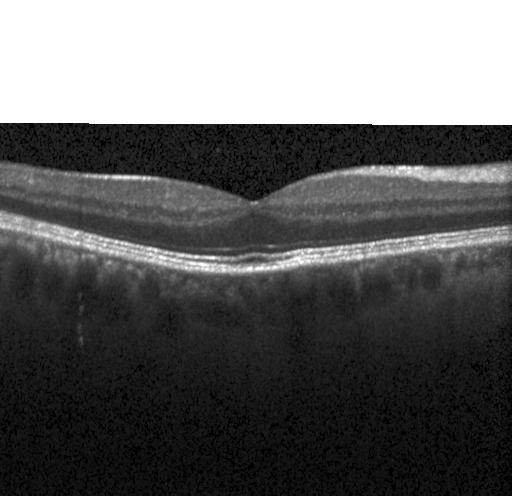 OCT B-scan showing neither CNV, DME, nor drusen.